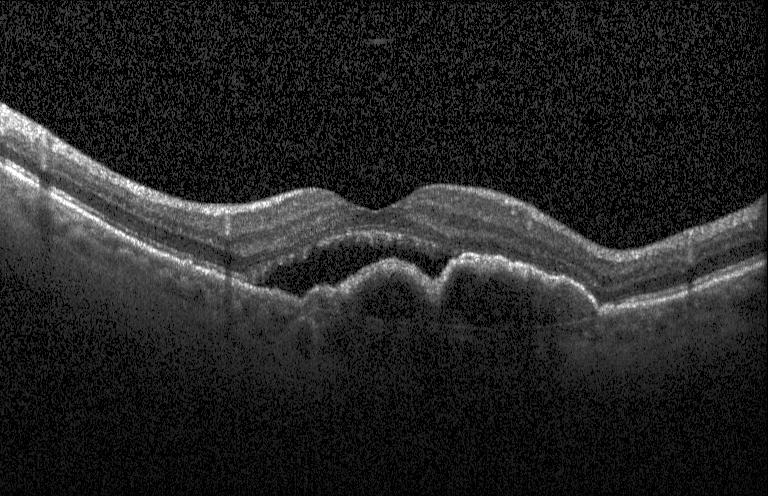 OCT line scan; spectral-domain OCT; fovea-centered; instrument: Heidelberg Spectralis. Choroidal neovascularization (CNV).